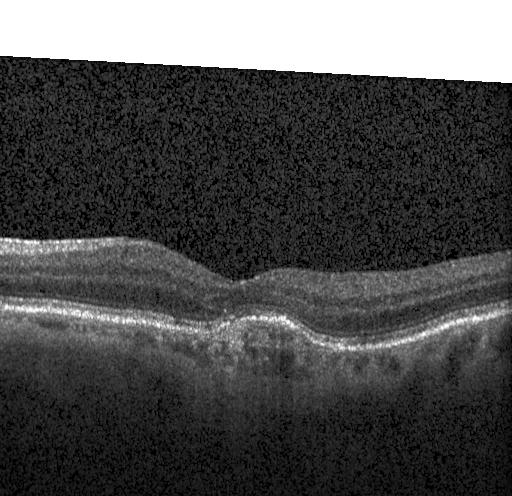 This B-scan demonstrates choroidal neovascularization.